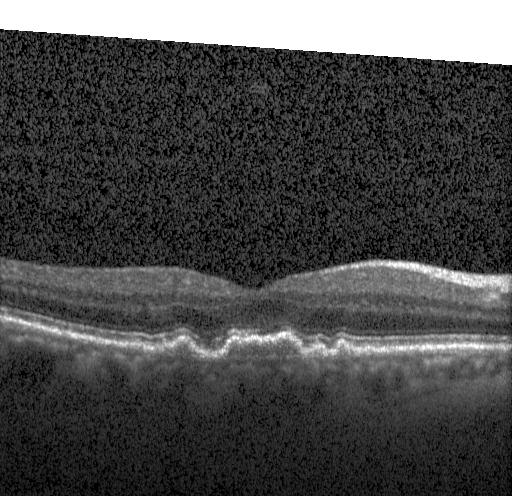

Through the macula; retinal OCT cross-section; spectral-domain OCT. Impression: a choroidal neovascular membrane.